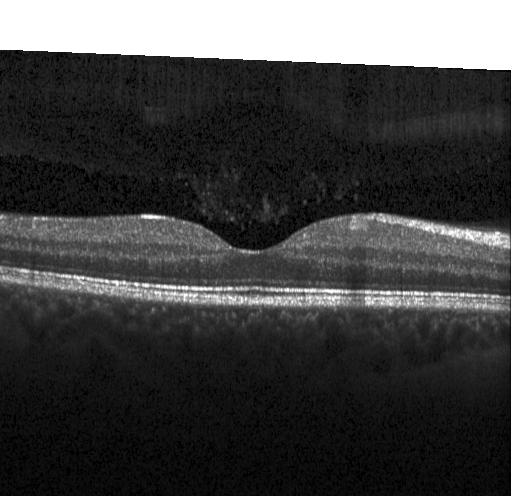

Finding: no evidence of choroidal neovascularization, diabetic macular edema, or drusen.